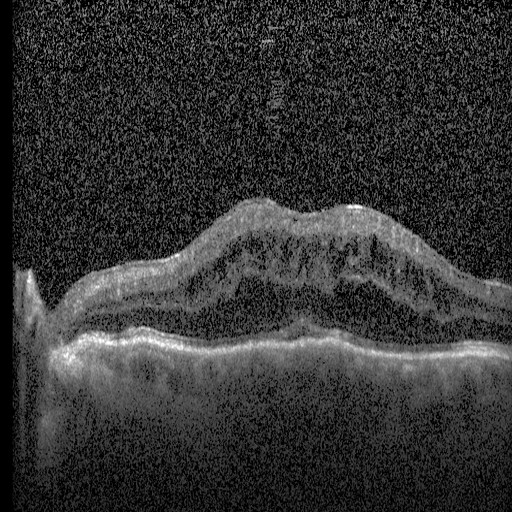
Optical coherence tomography scan — Finding: DME.